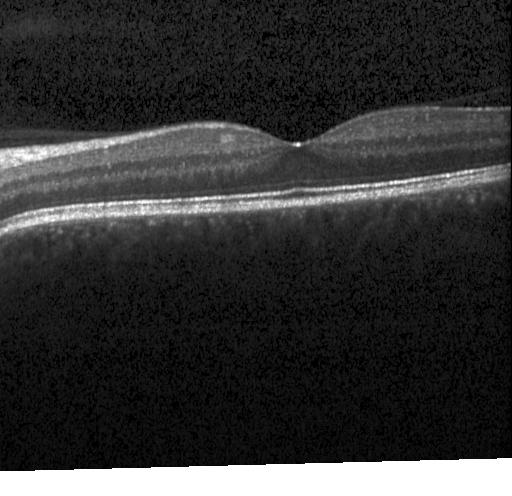

Spectral-domain optical coherence tomography. Optical coherence tomography scan. Centered on the fovea
No choroidal neovascularization, diabetic macular edema, or drusen.